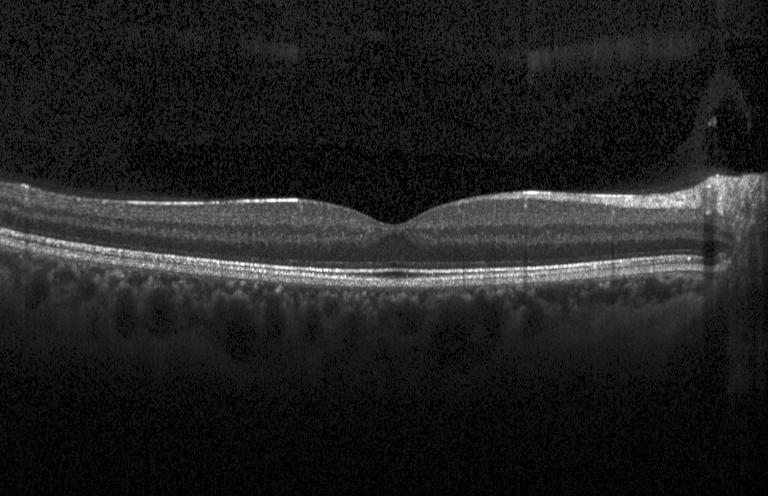
Retinal OCT cross-section, acquired on a Heidelberg Spectralis
Dx: no CNV, DME, or drusen.